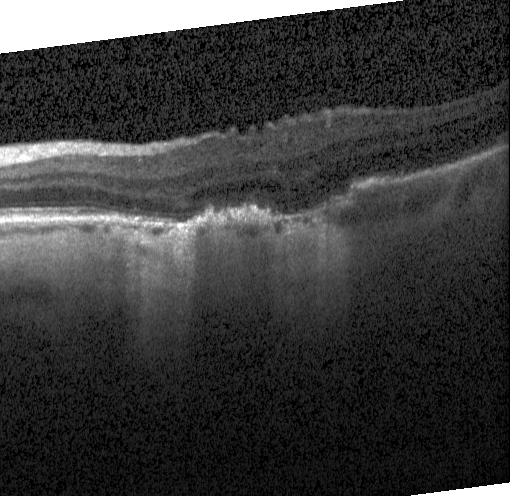
Diagnosis: CNV.